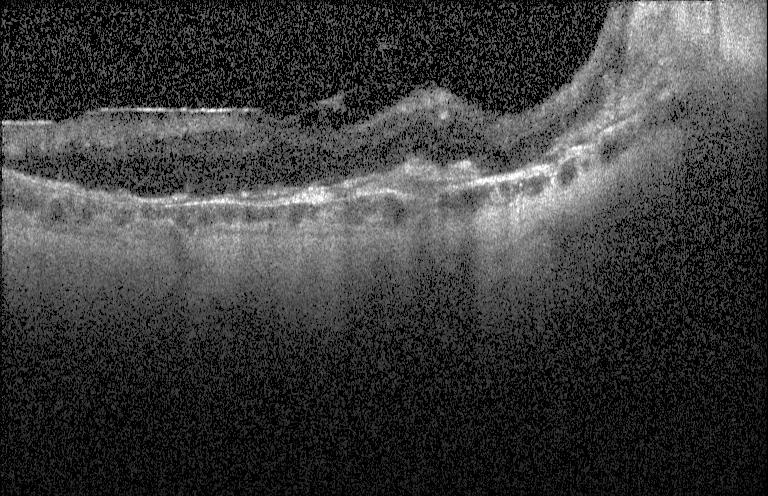

Spectral-domain optical coherence tomography · acquired on a Heidelberg Spectralis · through the macula · OCT B-scan. Impression: choroidal neovascularization.